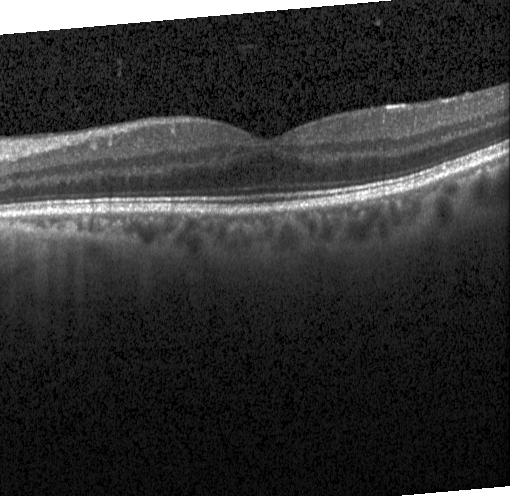 OCT scan showing neither choroidal neovascularization, diabetic macular edema, nor drusen.